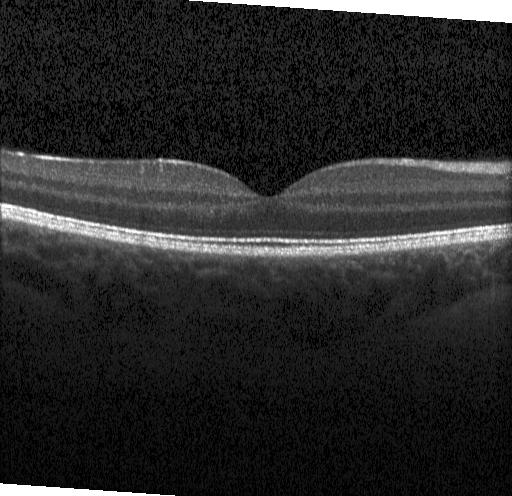 Impression: no choroidal neovascularization, no diabetic macular edema, and no drusen.